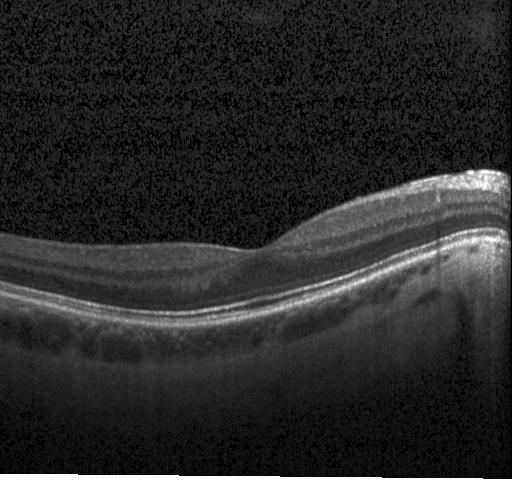
OCT line scan
Finding: no evidence of choroidal neovascularization, diabetic macular edema, or drusen.